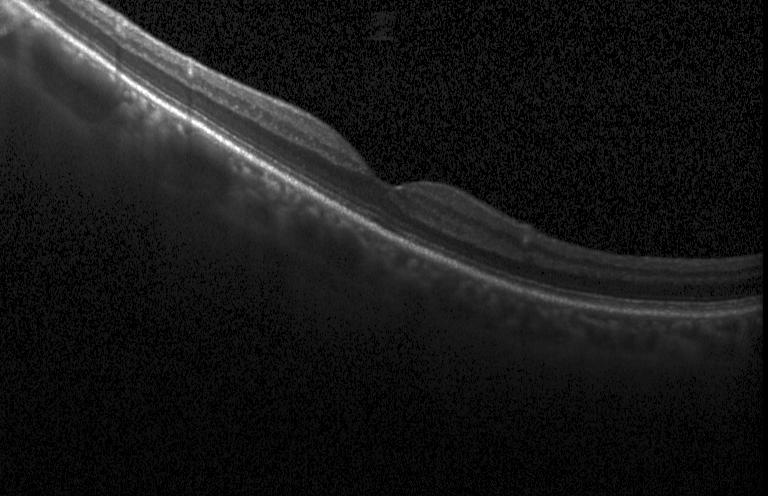 Instrument: Heidelberg Spectralis. Spectral-domain OCT. Retinal OCT B-scan. Finding: no evidence of CNV, DME, or drusen.